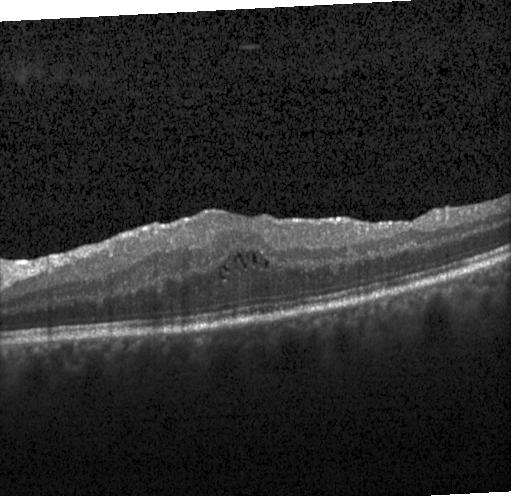

OCT line scan · instrument: Heidelberg Spectralis · macular scan
Impression: diabetic macular edema.